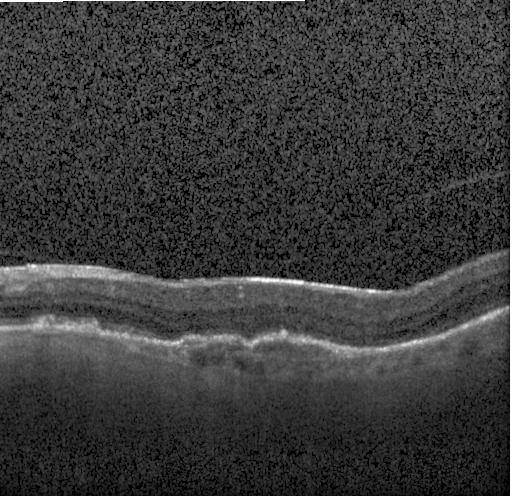

Centered on the fovea; SD-OCT; Heidelberg Spectralis; OCT line scan — Finding: choroidal neovascularization (CNV).